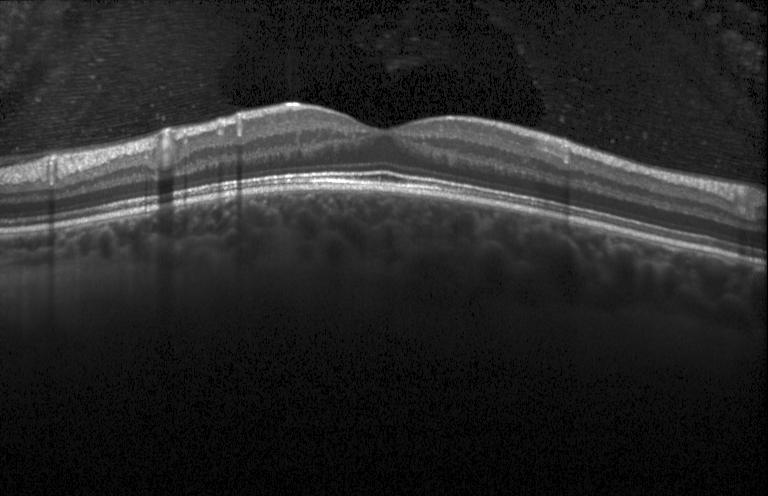 Diagnosis: no choroidal neovascularization, diabetic macular edema, or drusen.